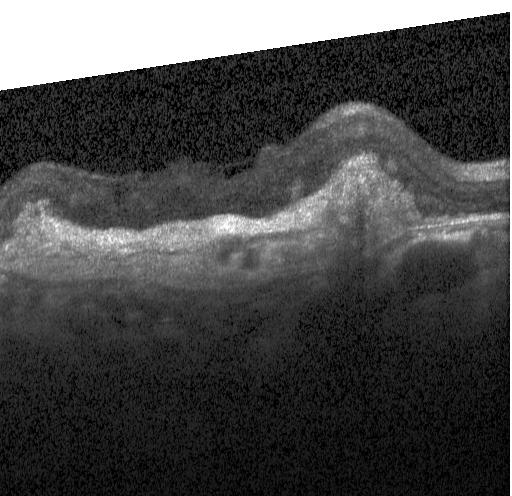

Spectral-domain OCT · optical coherence tomography scan. The scan shows a choroidal neovascular membrane.